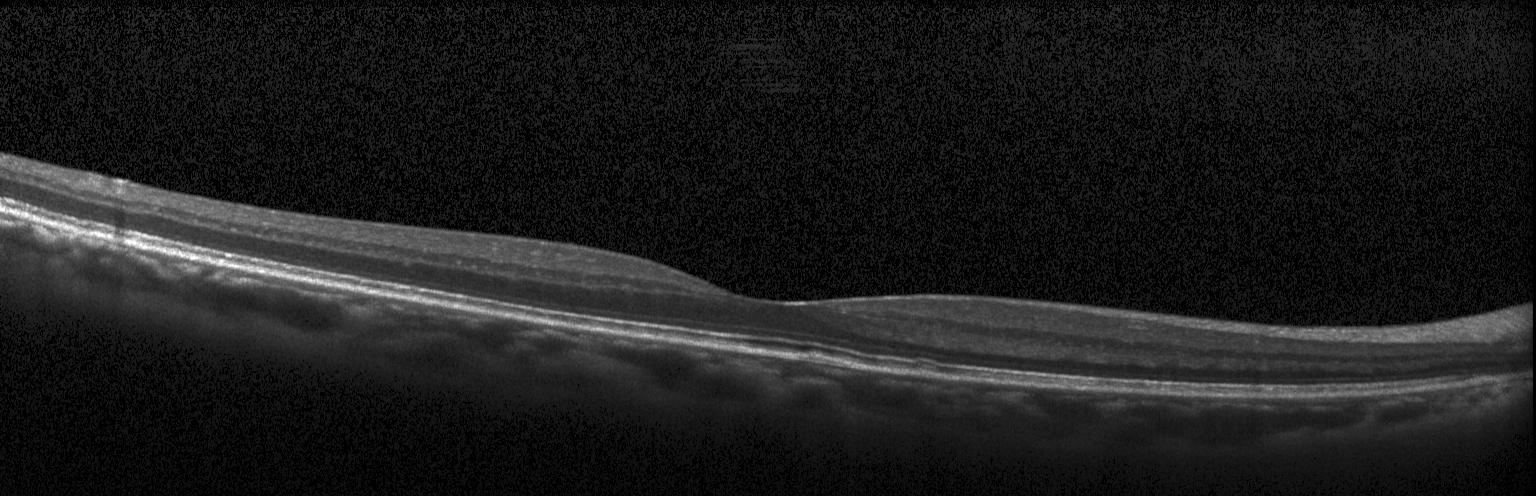

OCT scan showing no choroidal neovascularization, diabetic macular edema, or drusen.